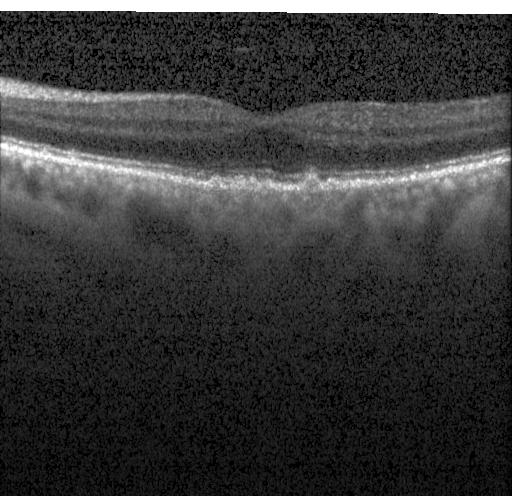
OCT B-scan; Heidelberg Spectralis OCT system.
The scan shows drusen.